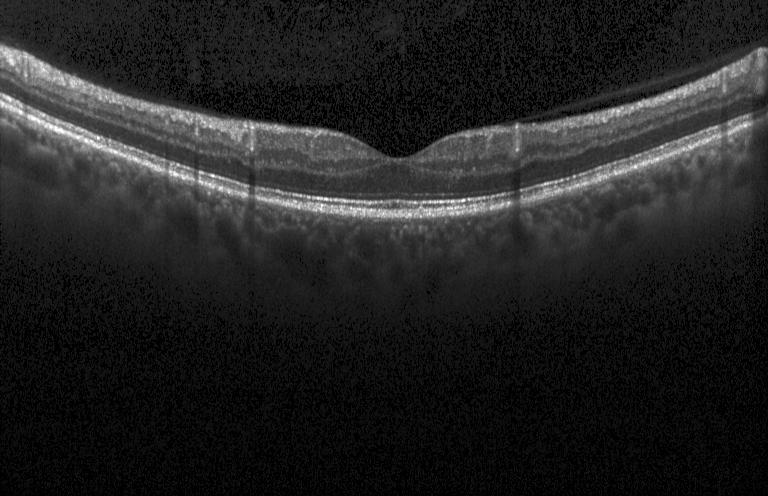
Impression: no choroidal neovascularization, diabetic macular edema, or drusen.